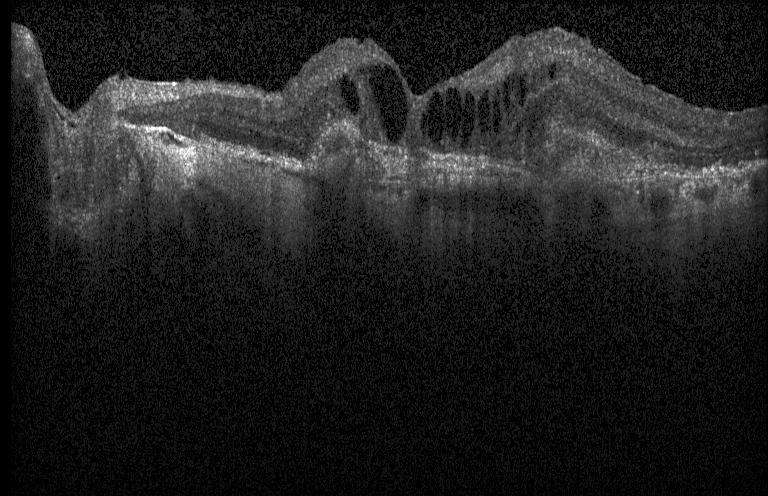

Heidelberg Spectralis, retinal OCT B-scan
Diagnosis: a choroidal neovascular membrane.